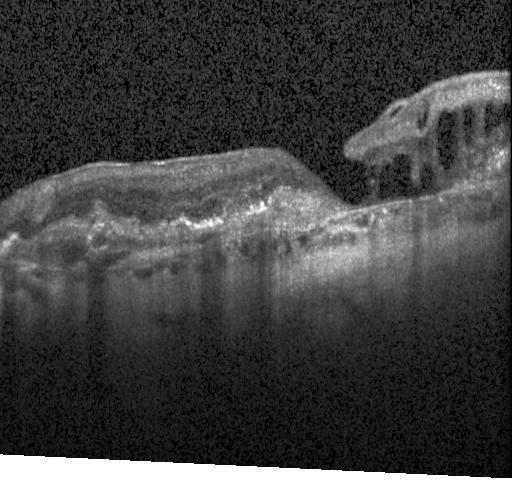 Horizontal scan through the fovea · retinal OCT B-scan · spectral-domain optical coherence tomography — Diagnosis: a choroidal neovascular membrane.